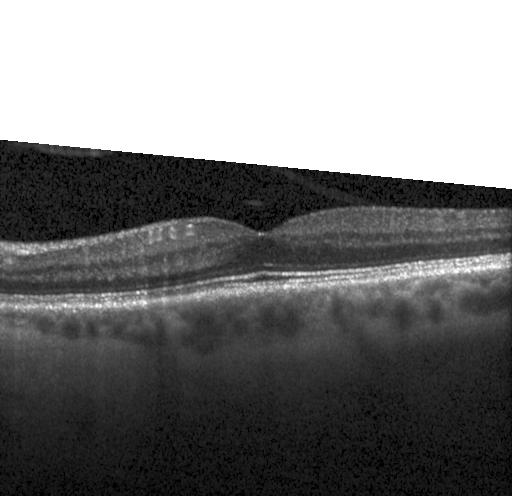 Dx: no CNV, no DME, and no drusen.